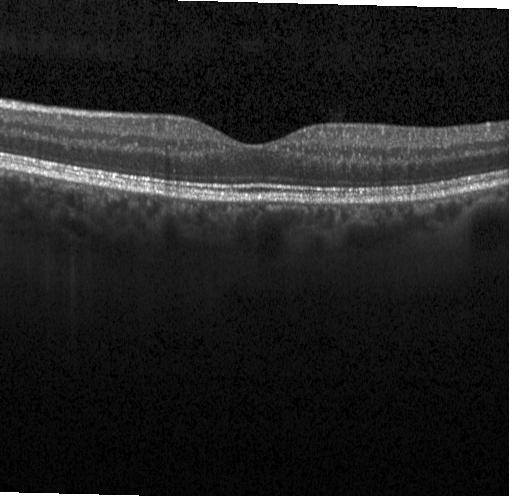
Acquired on a Heidelberg Spectralis. Through the macula. SD-OCT. Optical coherence tomography B-scan
Dx: neither CNV, DME, nor drusen.